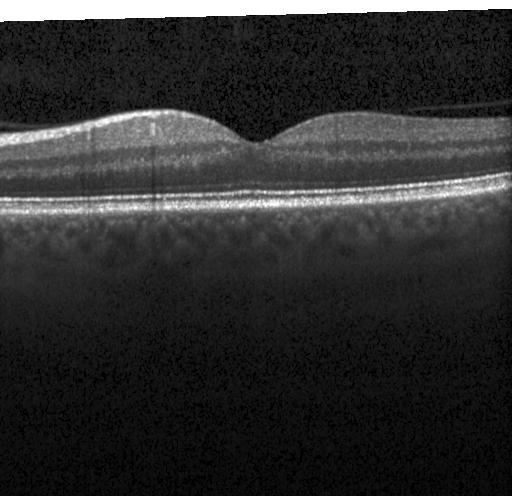

Optical coherence tomography scan; fovea-centered — Impression: no evidence of choroidal neovascularization, diabetic macular edema, or drusen.